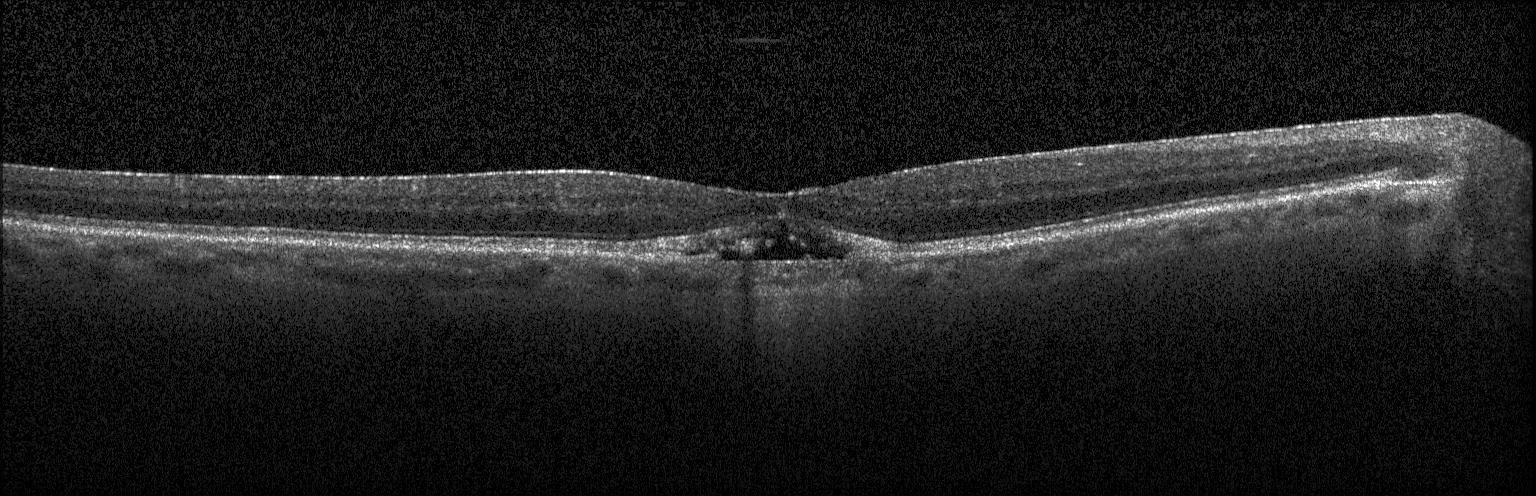

Diagnosis: a choroidal neovascular membrane.